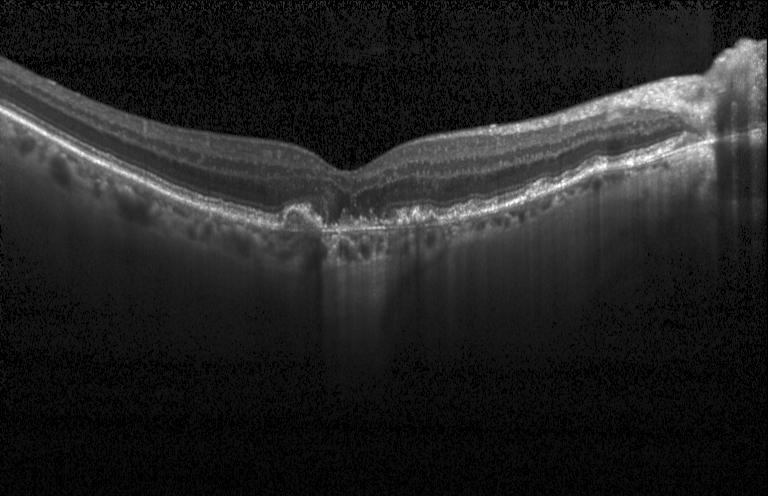
Macular OCT demonstrating a choroidal neovascular membrane.